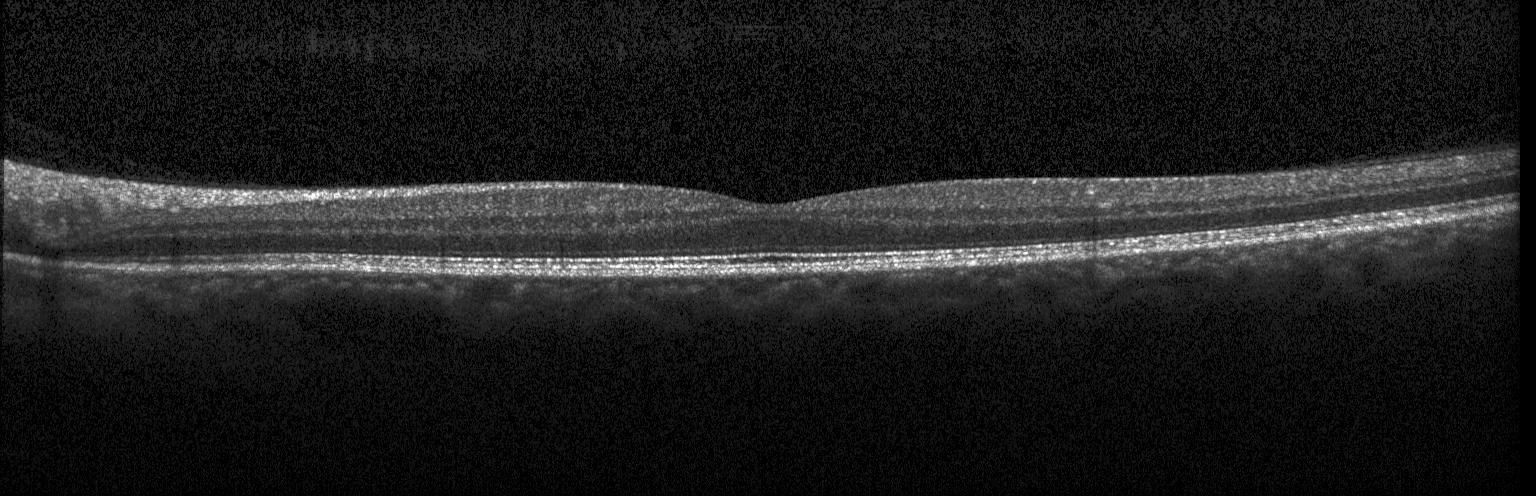

OCT finding: no CNV, no DME, and no drusen.